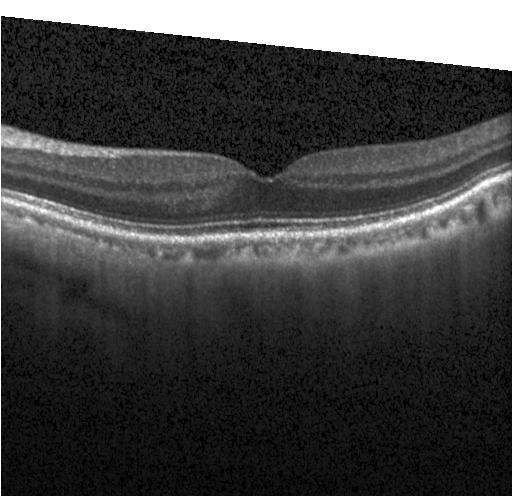
Retinal OCT B-scan. Spectral-domain OCT. Centered on the fovea
Finding: no choroidal neovascularization, diabetic macular edema, or drusen.